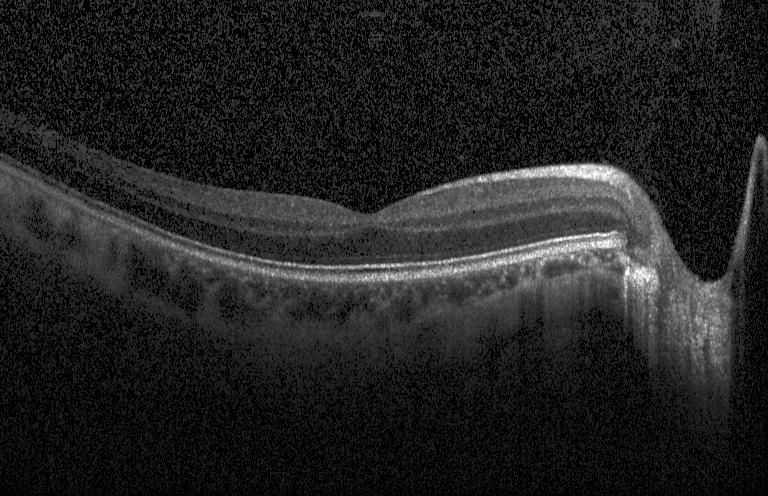
Assessment: no evidence of choroidal neovascularization, diabetic macular edema, or drusen.